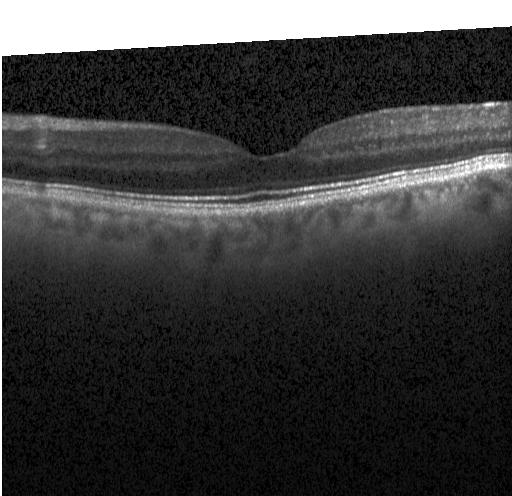 Dx: neither CNV, DME, nor drusen.